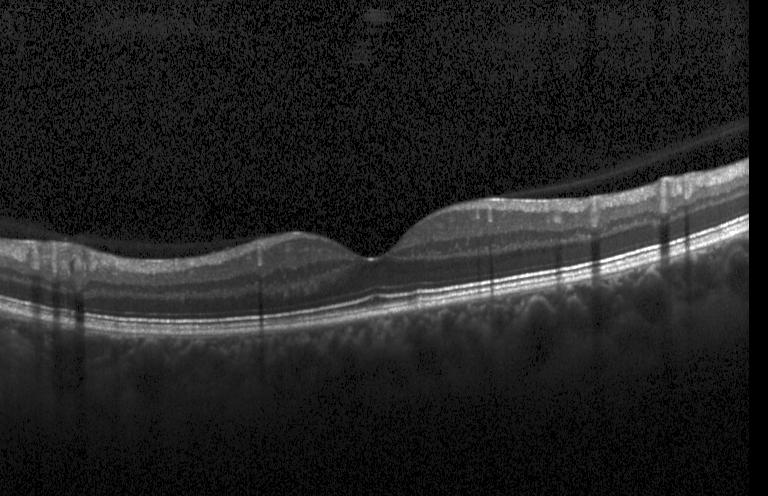 Spectral-domain optical coherence tomography, instrument: Heidelberg Spectralis, optical coherence tomography B-scan, fovea-centered.
Assessment: no evidence of choroidal neovascularization, diabetic macular edema, or drusen.